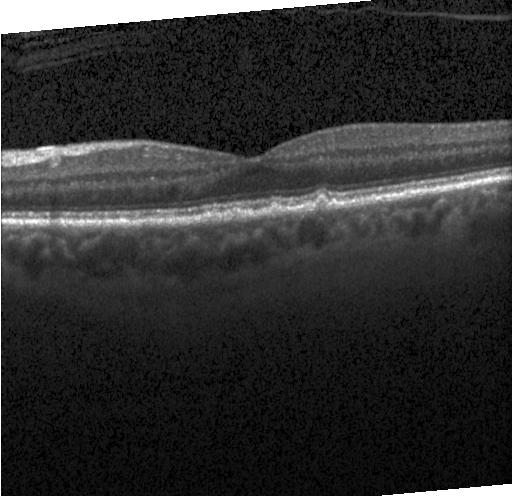

Retinal OCT cross-section showing sub-RPE drusenoid deposits.